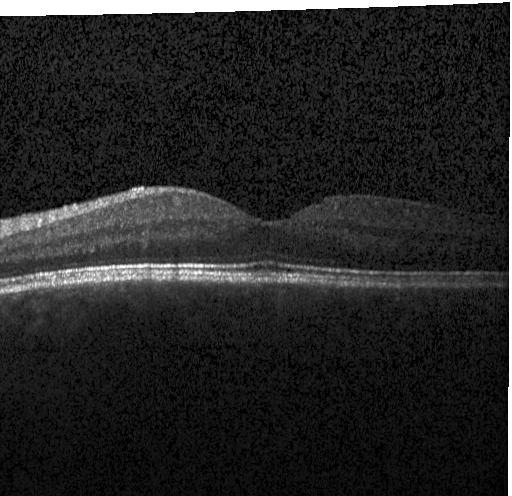

Centered on the fovea; optical coherence tomography B-scan — Finding: no CNV, no DME, and no drusen.